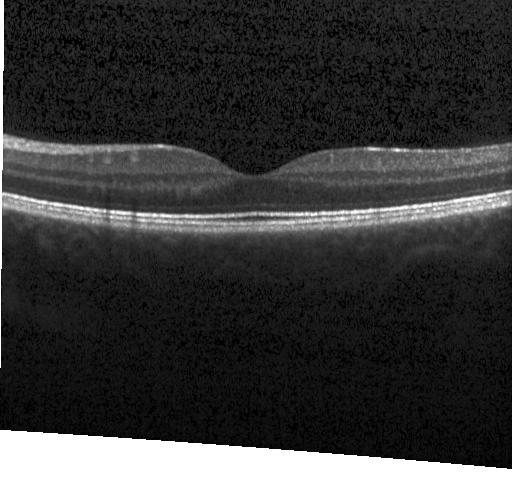
OCT B-scan, spectral-domain optical coherence tomography, horizontal scan through the fovea, instrument: Heidelberg Spectralis.
The scan shows no choroidal neovascularization, diabetic macular edema, or drusen.